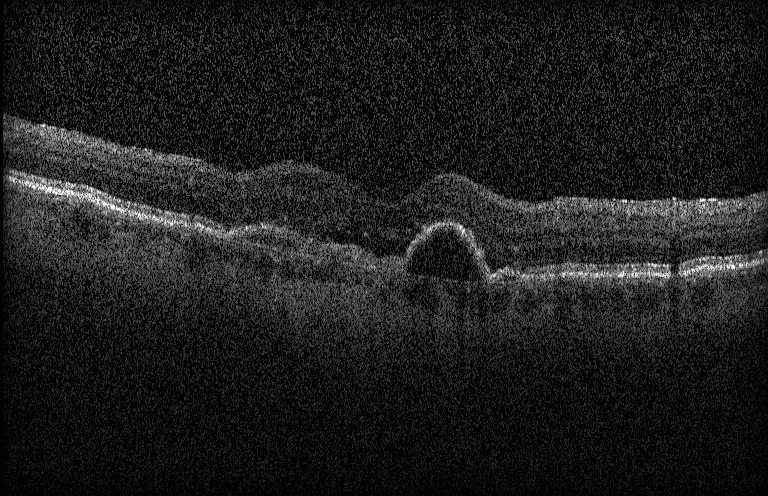

Optical coherence tomography scan.
Finding: a choroidal neovascular membrane.